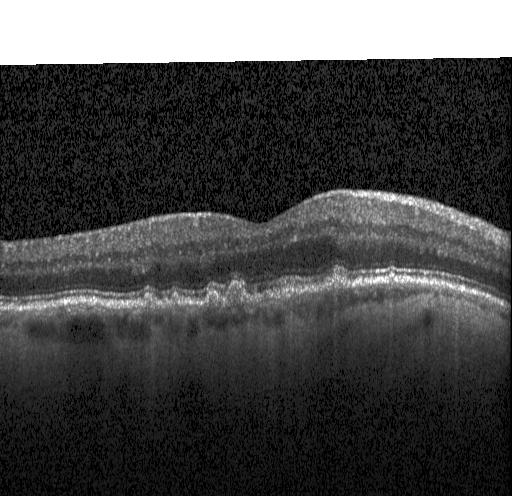 Finding: multiple drusen.